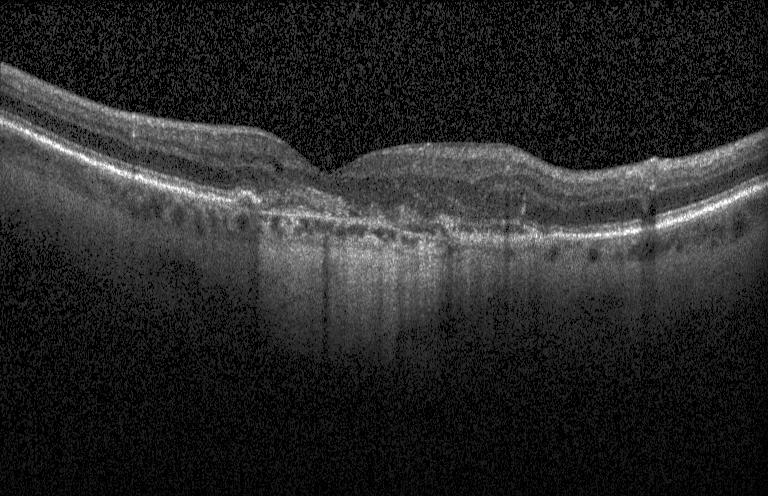 Retinal OCT B-scan; spectral-domain optical coherence tomography; through the macula — Macular OCT: a choroidal neovascular membrane.